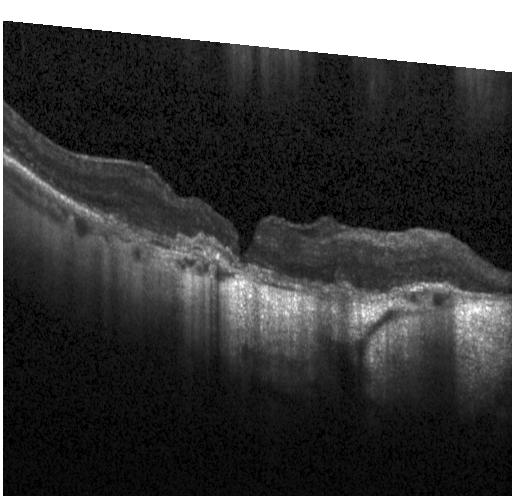
Fovea-centered · Heidelberg Spectralis OCT system · retinal OCT B-scan
Dx: a choroidal neovascular membrane.